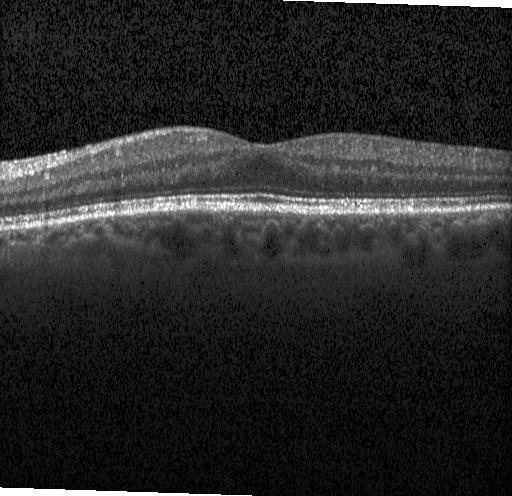

Heidelberg Spectralis OCT system · OCT B-scan · SD-OCT.
Finding: no choroidal neovascularization, diabetic macular edema, or drusen.